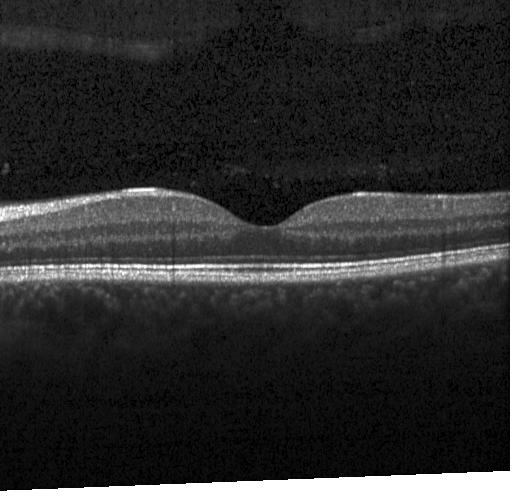
Dx: no CNV, no DME, and no drusen.